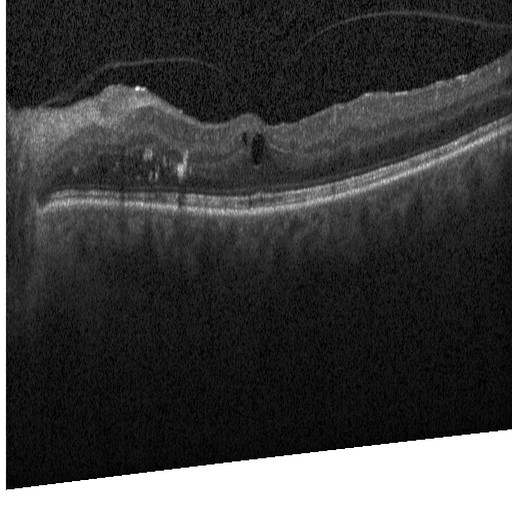
Instrument: Heidelberg Spectralis, optical coherence tomography B-scan, spectral-domain optical coherence tomography.
Impression: diabetic macular edema.